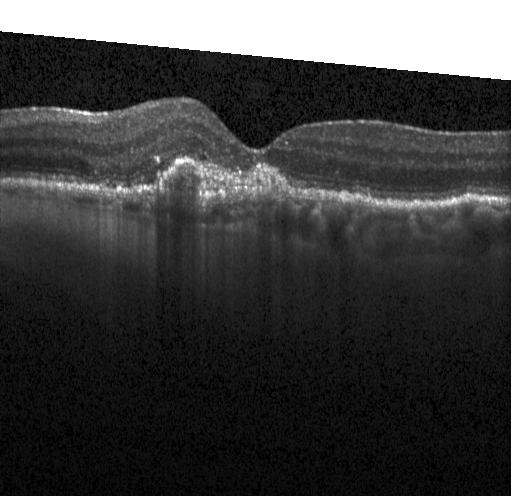 OCT B-scan, Heidelberg Spectralis OCT system, macular scan
Assessment: a choroidal neovascular membrane.